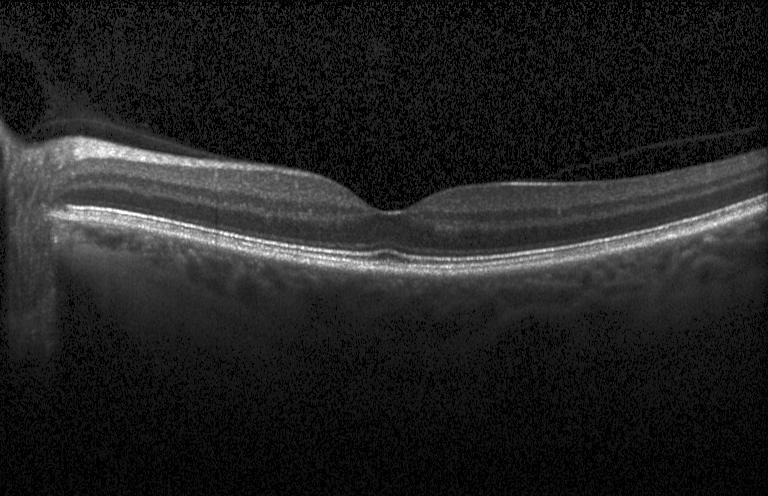 Retinal OCT B-scan, Heidelberg Spectralis OCT system, through the macula, spectral-domain optical coherence tomography
Dx: neither choroidal neovascularization, diabetic macular edema, nor drusen.